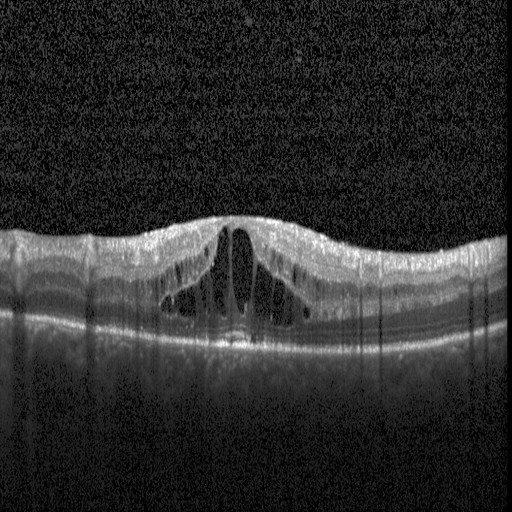

Instrument: Heidelberg Spectralis; SD-OCT; retinal OCT B-scan; horizontal scan through the fovea.
Finding: diabetic macular edema (DME).